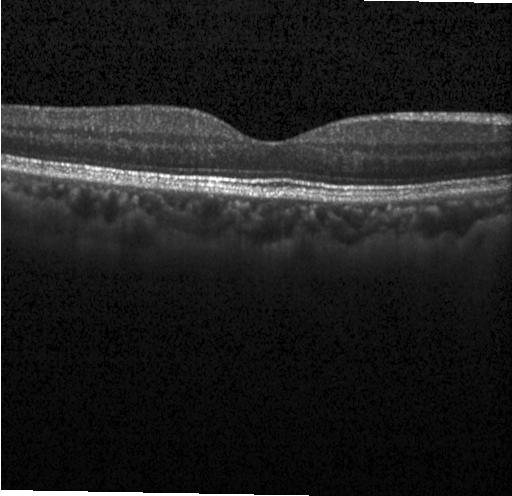

Heidelberg Spectralis; macular scan; optical coherence tomography scan. OCT finding: no CNV, DME, or drusen.